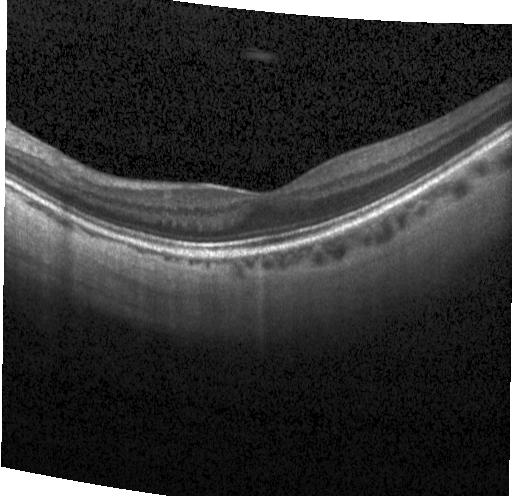
OCT B-scan. SD-OCT
Diagnosis: no choroidal neovascularization, no diabetic macular edema, and no drusen.